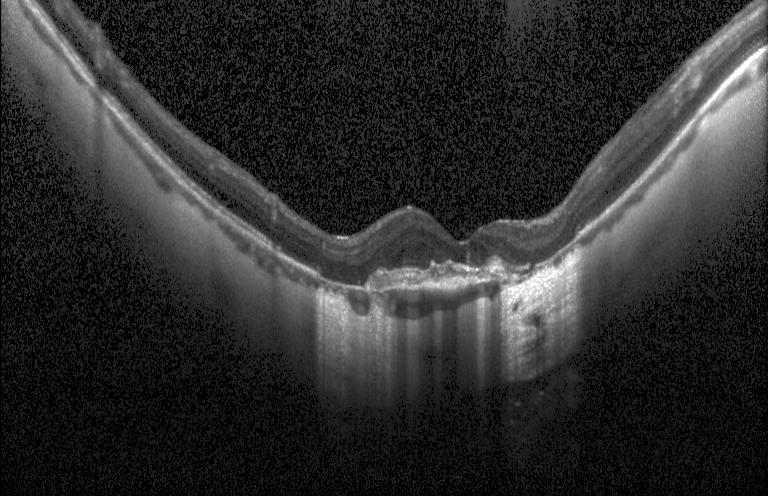
Finding: a choroidal neovascular membrane.